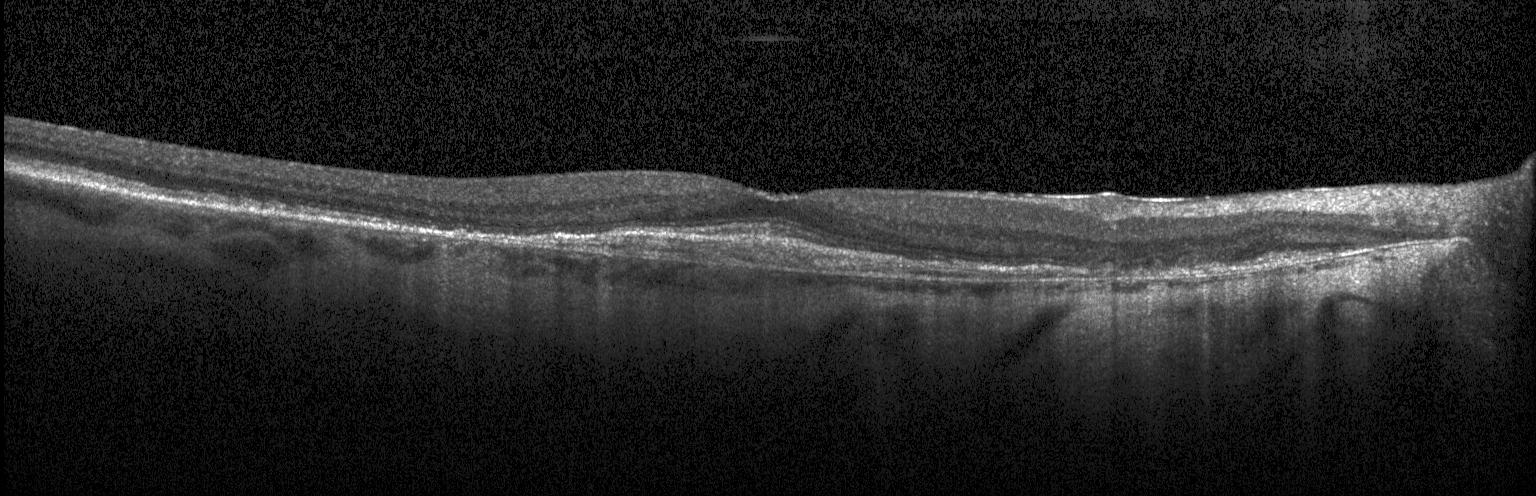 OCT B-scan. Finding: a choroidal neovascular membrane.